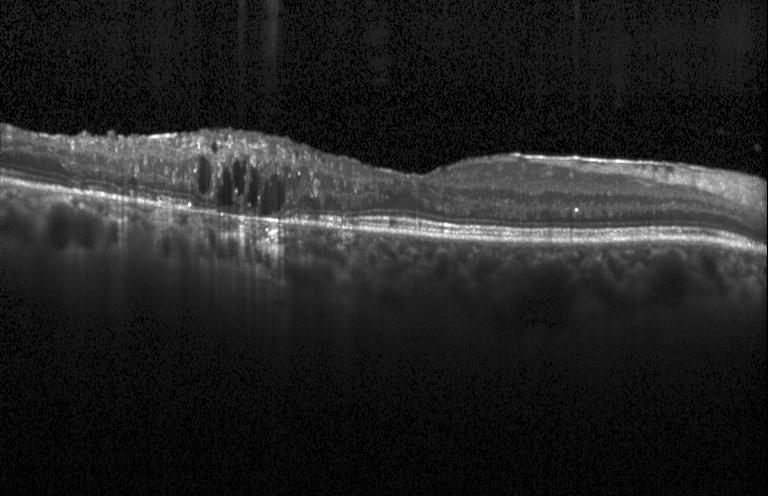

Heidelberg Spectralis. Optical coherence tomography scan. Spectral-domain OCT. Macular scan — Diagnosis: DME.